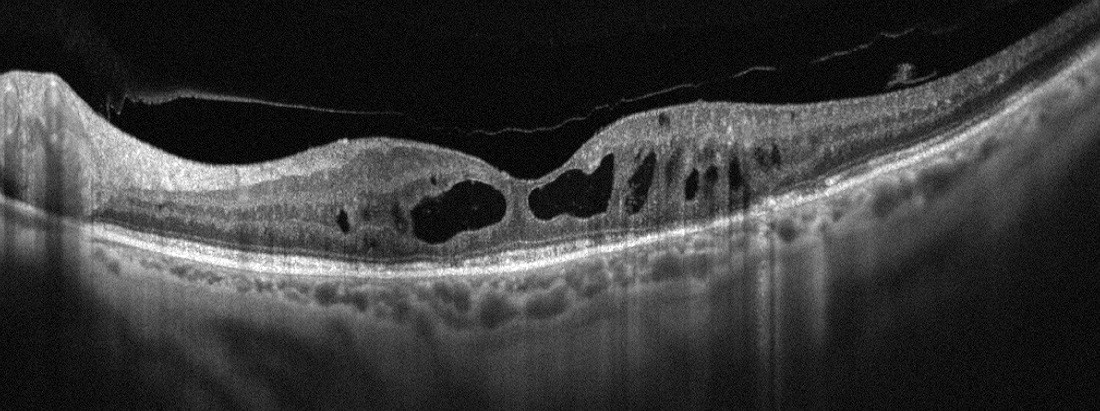

Retinal OCT cross-section showing diabetic macular edema.